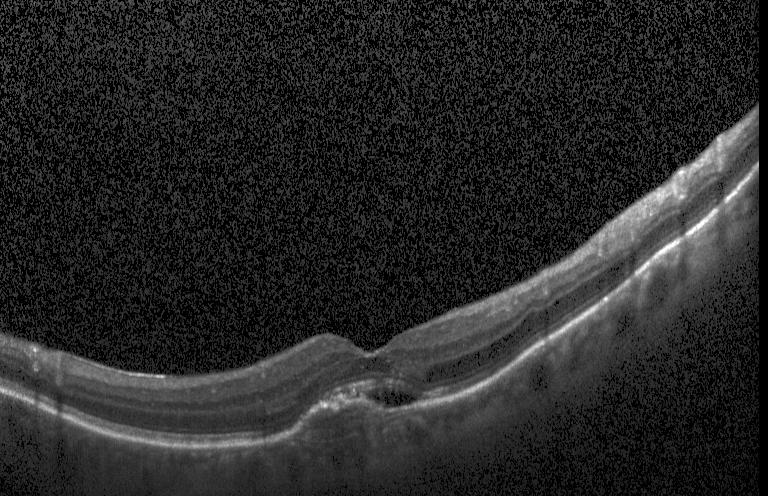
OCT B-scan. Heidelberg Spectralis. SD-OCT.
This B-scan demonstrates CNV.